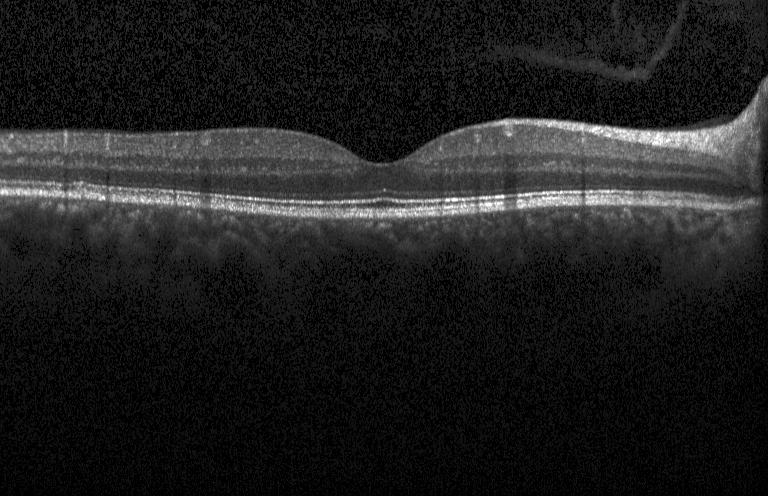
This B-scan demonstrates no evidence of choroidal neovascularization, diabetic macular edema, or drusen.